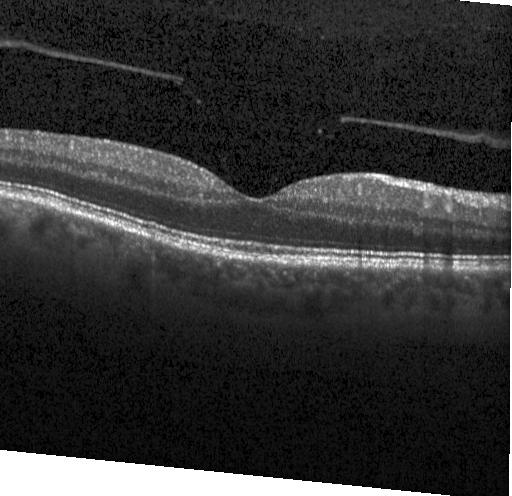 OCT B-scan.
Assessment: no choroidal neovascularization, diabetic macular edema, or drusen.